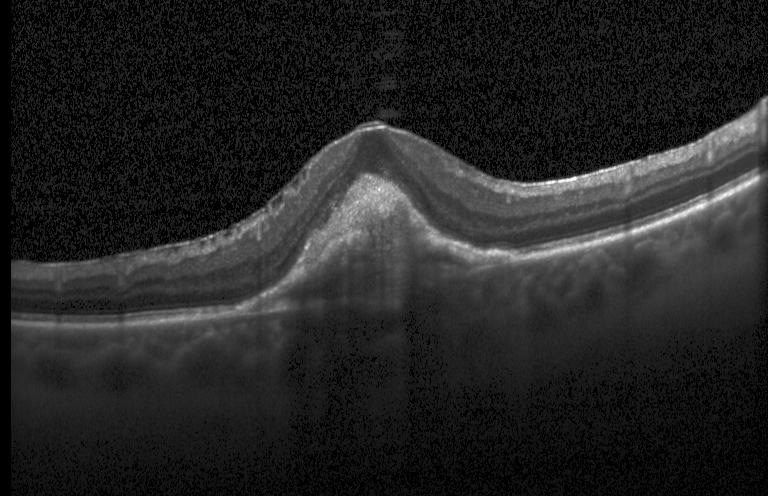 A choroidal neovascular membrane.